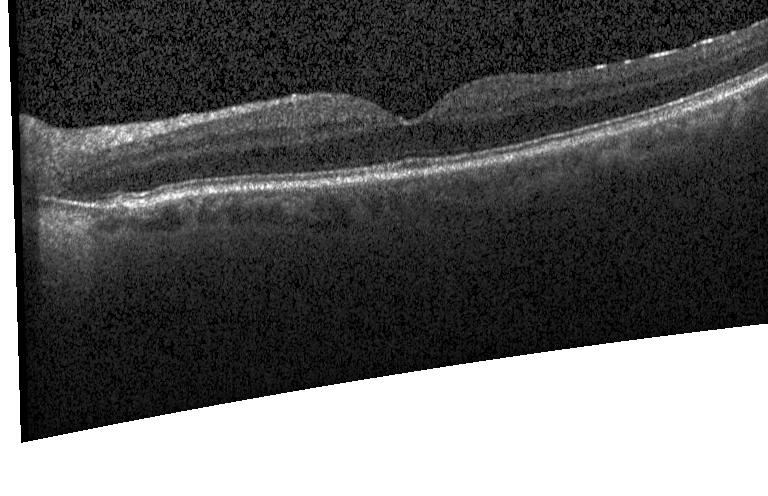
Heidelberg Spectralis OCT system, retinal OCT B-scan, through the macula — Diagnosis: no evidence of CNV, DME, or drusen.